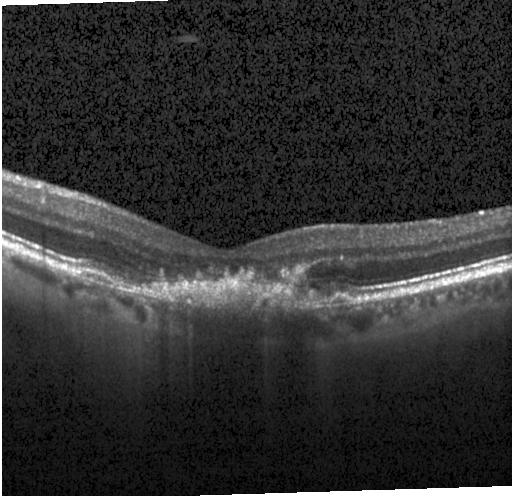
Optical coherence tomography B-scan. Finding: a choroidal neovascular membrane.